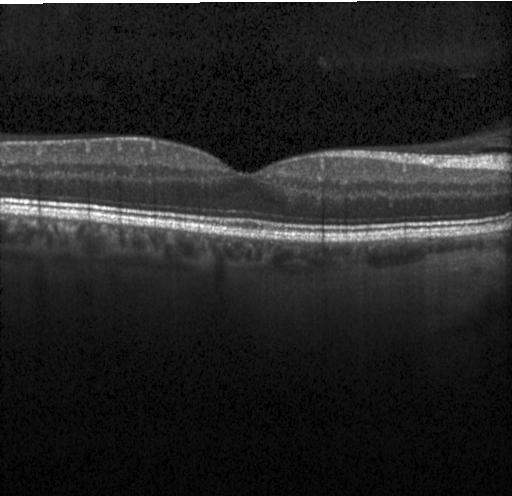
Retinal OCT cross-section. Acquired on a Heidelberg Spectralis. Fovea-centered
Finding: neither choroidal neovascularization, diabetic macular edema, nor drusen.